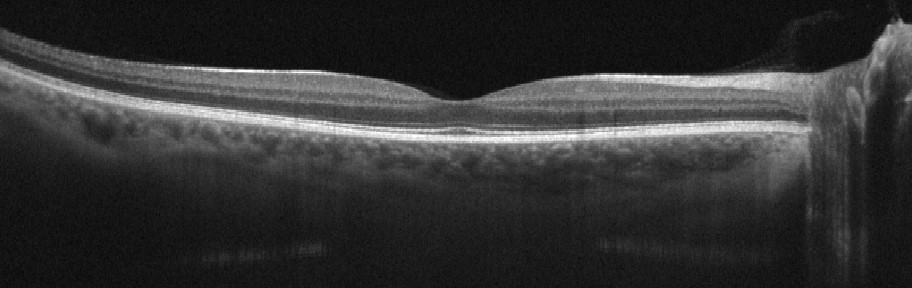

Retinal OCT B-scan. Finding: no AMD, DME, ERM, RAO, RVO, or VID.